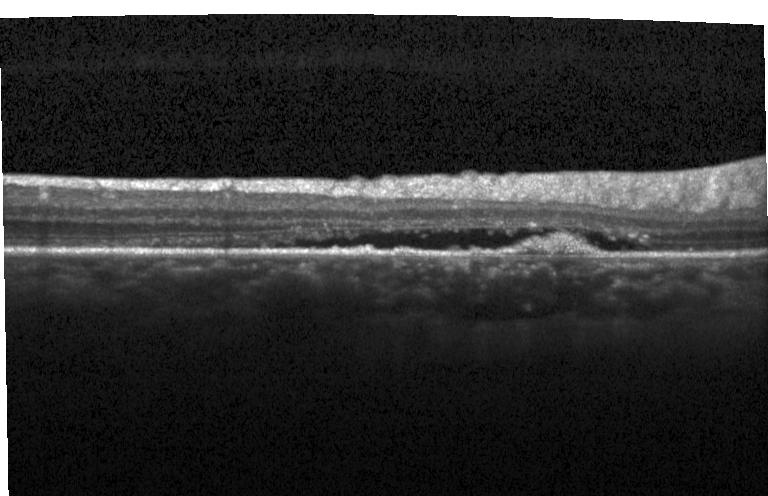 Macular OCT: choroidal neovascularization (CNV).